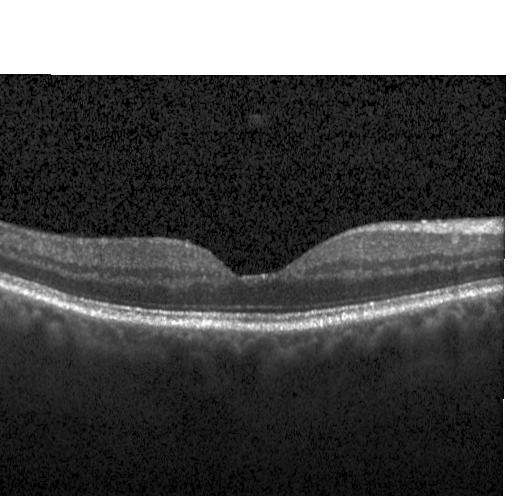
OCT B-scan — Diagnosis: no evidence of choroidal neovascularization, diabetic macular edema, or drusen.